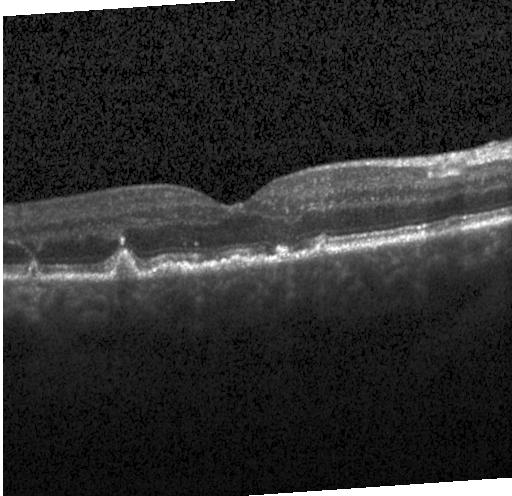

Acquired on a Heidelberg Spectralis. Retinal OCT B-scan. SD-OCT. Horizontal scan through the fovea
Impression: sub-RPE drusenoid deposits.